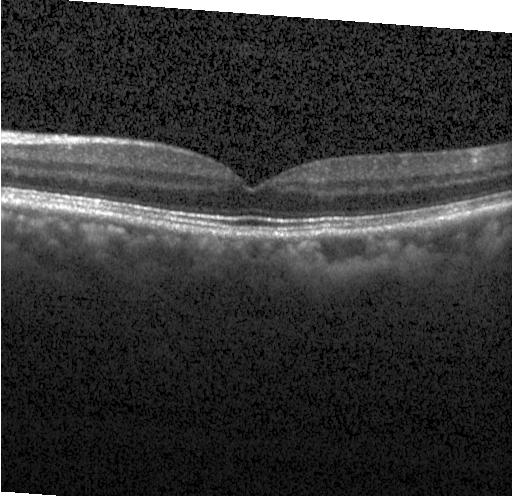
SD-OCT. Optical coherence tomography scan. Through the macula
This B-scan demonstrates neither choroidal neovascularization, diabetic macular edema, nor drusen.